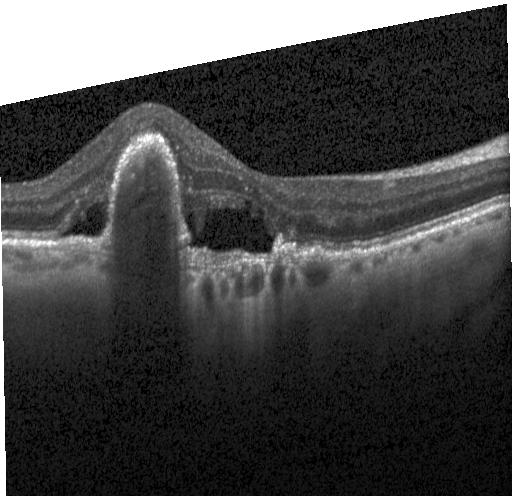
Retinal OCT cross-section. SD-OCT. Heidelberg Spectralis. Dx: a choroidal neovascular membrane.